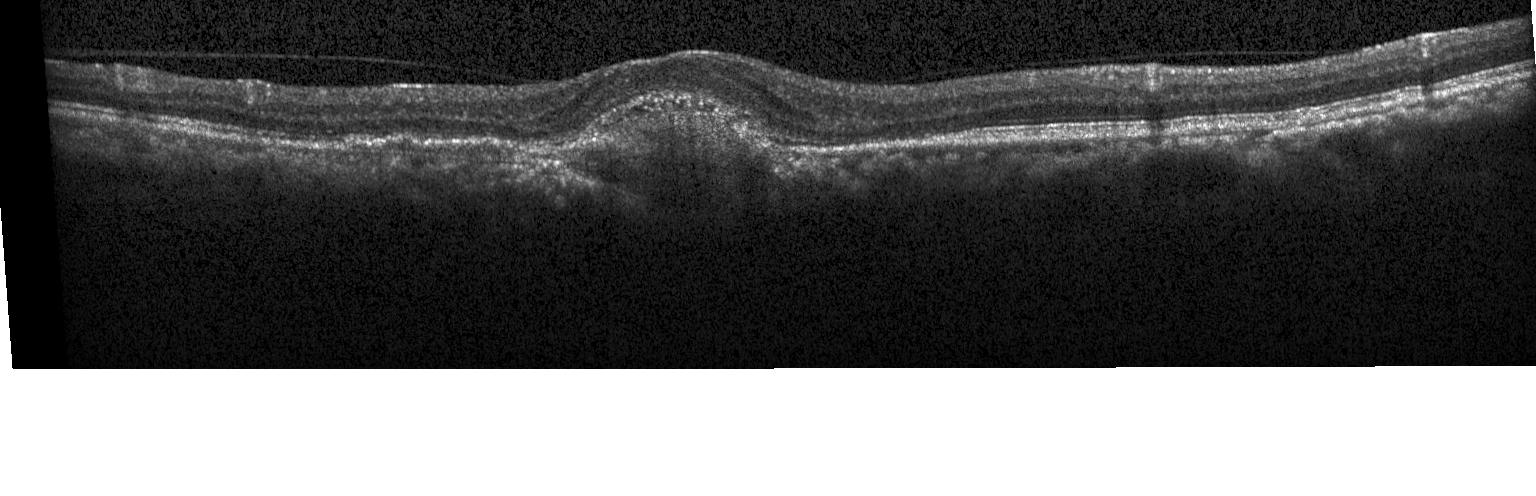

Macular OCT demonstrating a choroidal neovascular membrane.